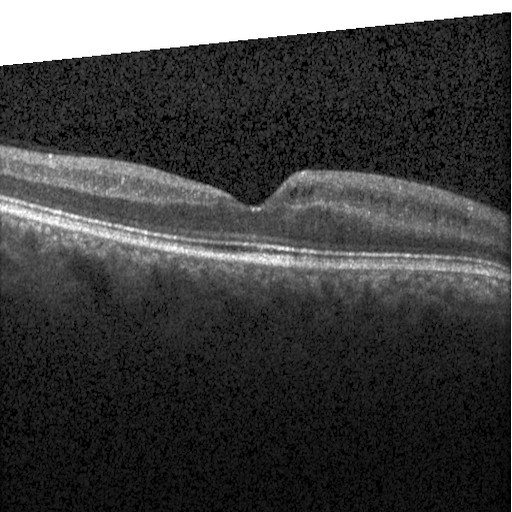
Finding: diabetic macular edema.